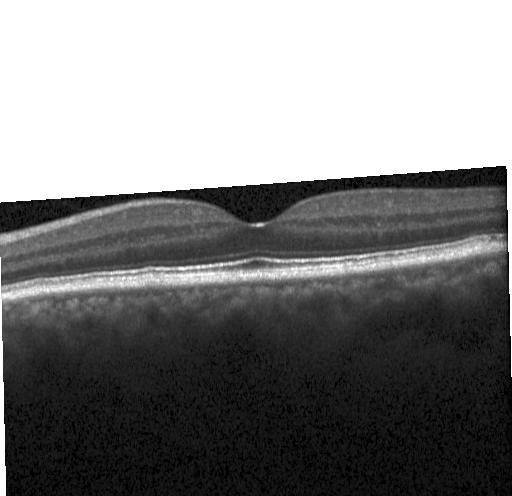 OCT B-scan — This B-scan demonstrates no evidence of choroidal neovascularization, diabetic macular edema, or drusen.